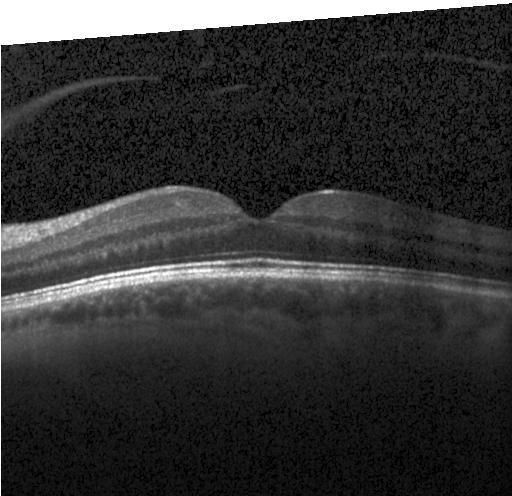 OCT finding: no CNV, no DME, and no drusen.